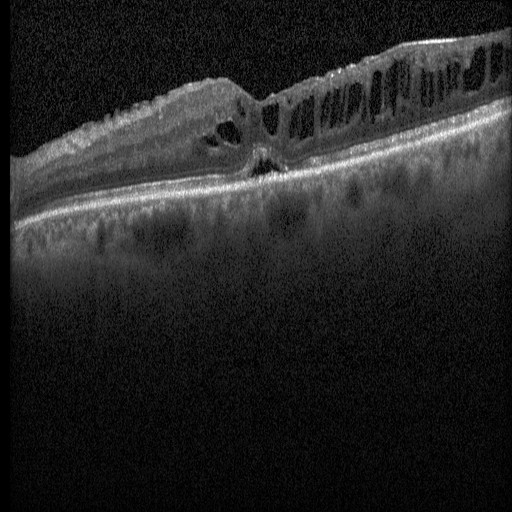 OCT B-scan — Finding: diabetic macular edema.